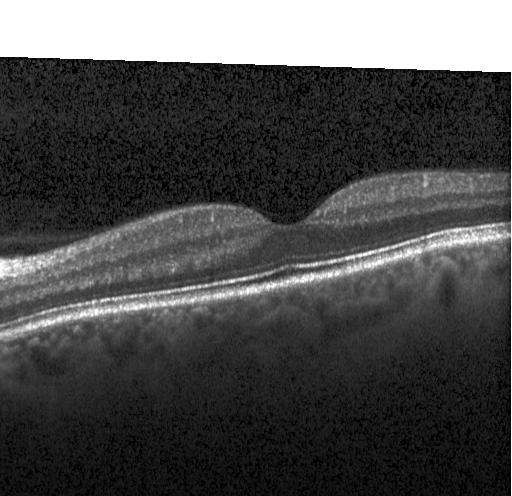

OCT scan showing no evidence of choroidal neovascularization, diabetic macular edema, or drusen.